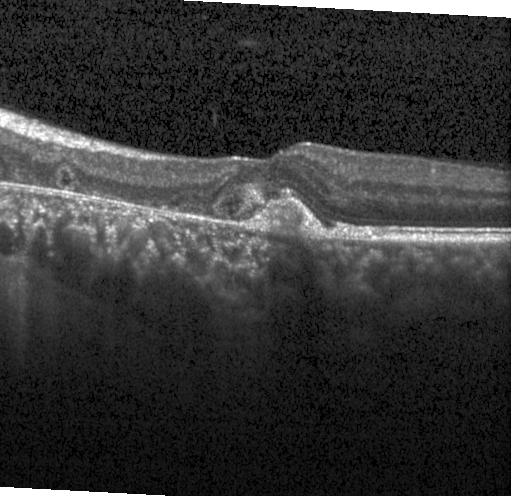

Macular scan, OCT B-scan, spectral-domain OCT, Heidelberg Spectralis.
Impression: CNV.